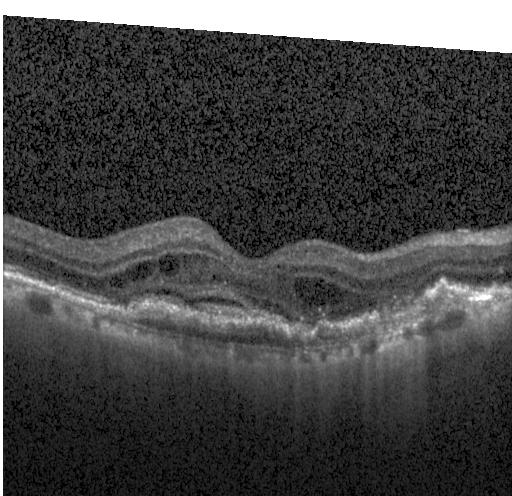
Impression: a choroidal neovascular membrane.